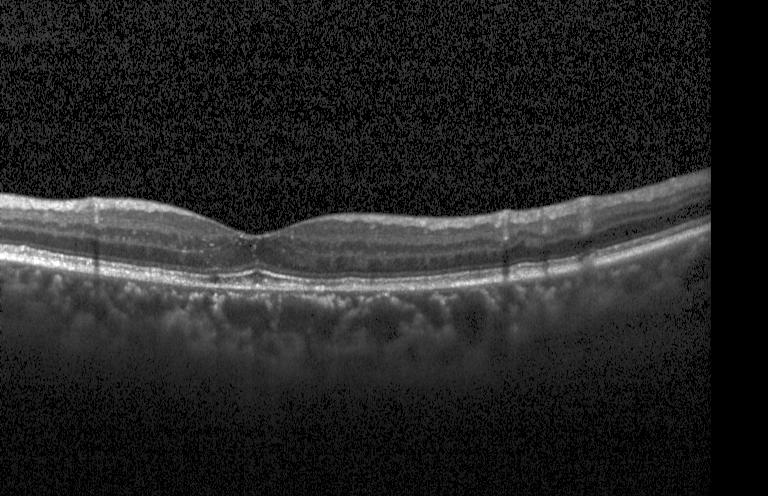 Retinal OCT B-scan
Finding: neither choroidal neovascularization, diabetic macular edema, nor drusen.